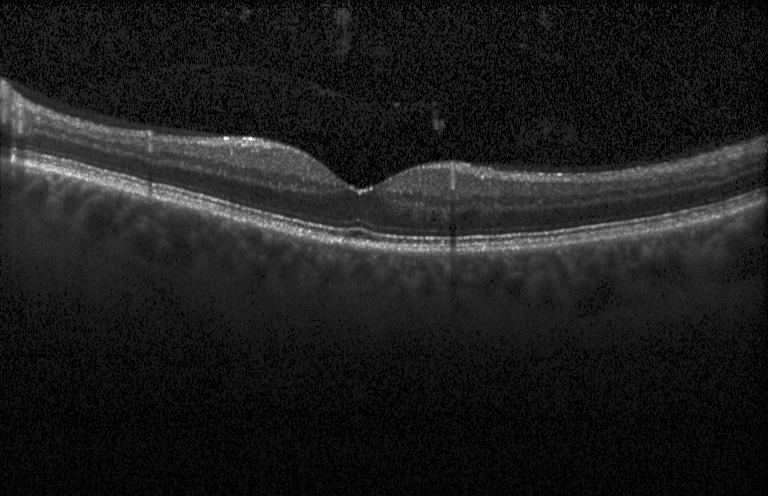
Instrument: Heidelberg Spectralis, spectral-domain optical coherence tomography, retinal OCT cross-section, macular scan
No evidence of choroidal neovascularization, diabetic macular edema, or drusen.